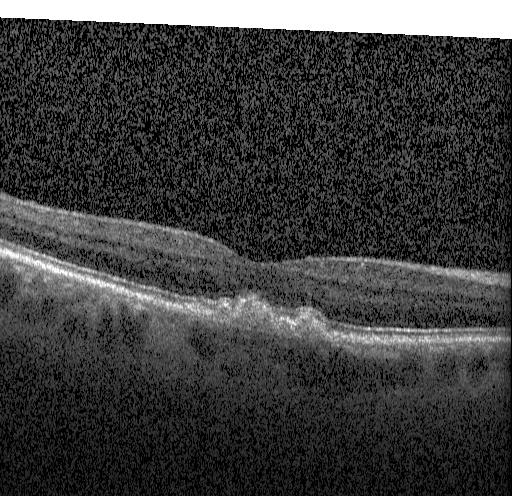 Retinal OCT cross-section showing sub-RPE drusenoid deposits.